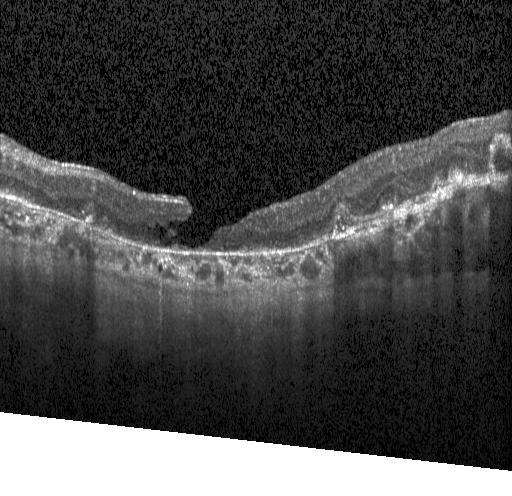 OCT B-scan. Through the macula.
Finding: a choroidal neovascular membrane.